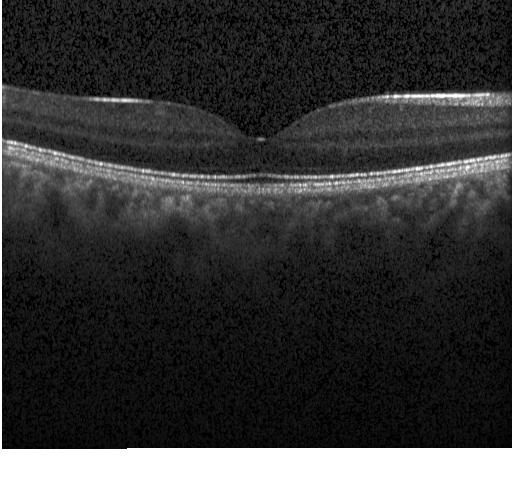 OCT line scan
Diagnosis: no CNV, DME, or drusen.